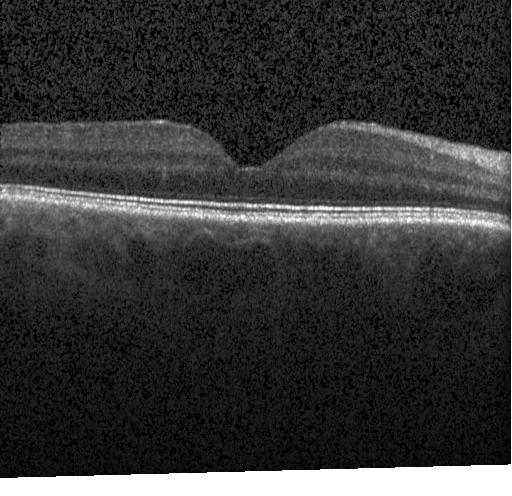

Instrument: Heidelberg Spectralis · optical coherence tomography scan · SD-OCT. Diagnosis: neither CNV, DME, nor drusen.